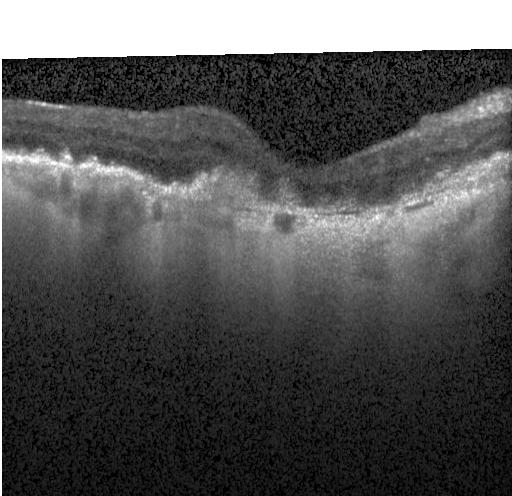
Diagnosis: a choroidal neovascular membrane.